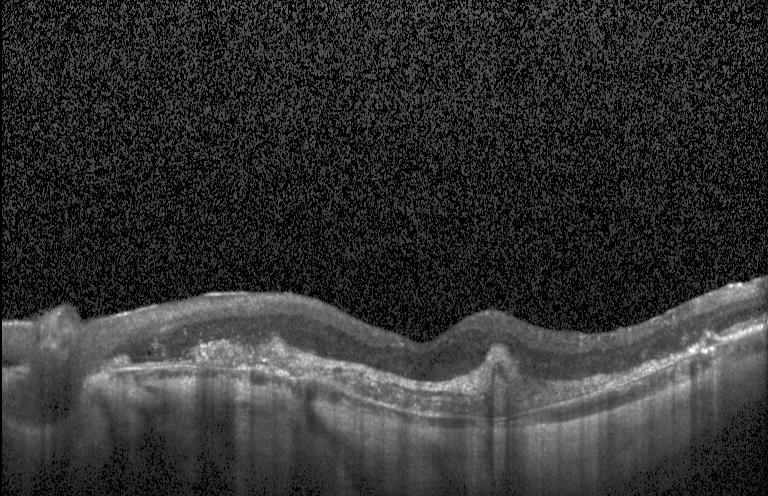

OCT finding: a choroidal neovascular membrane.